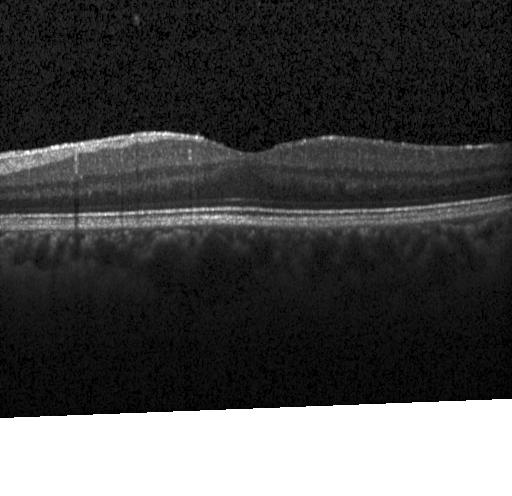 Assessment: no evidence of choroidal neovascularization, diabetic macular edema, or drusen.